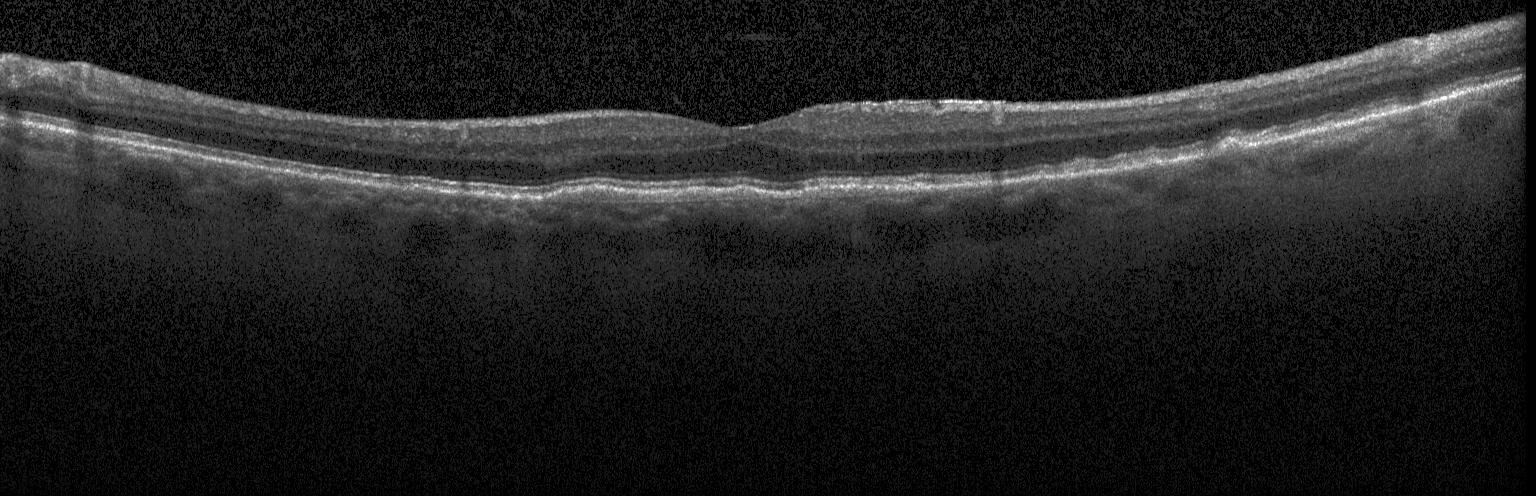 OCT line scan
Diagnosis: a choroidal neovascular membrane.